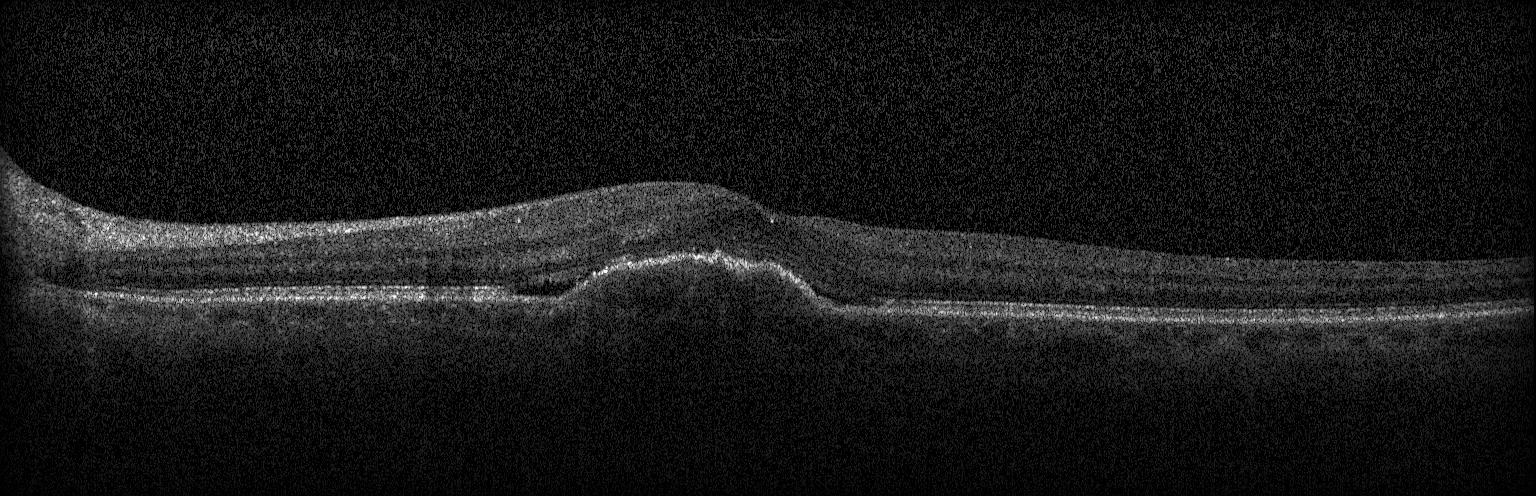 The scan shows choroidal neovascularization (CNV).